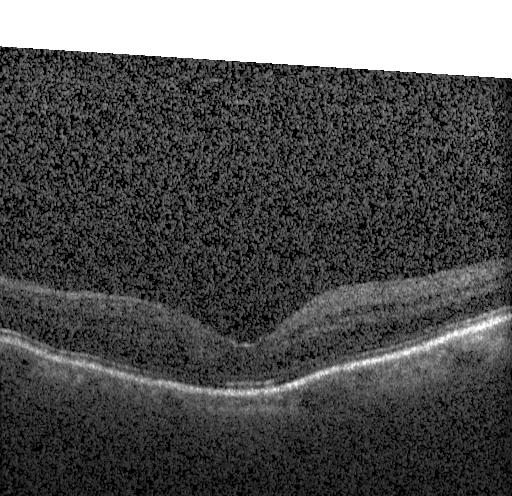 Centered on the fovea. Retinal OCT B-scan.
The scan shows neither CNV, DME, nor drusen.